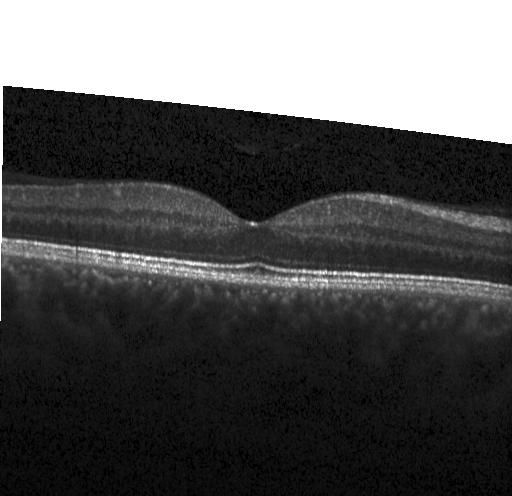
Optical coherence tomography scan — OCT finding: neither choroidal neovascularization, diabetic macular edema, nor drusen.